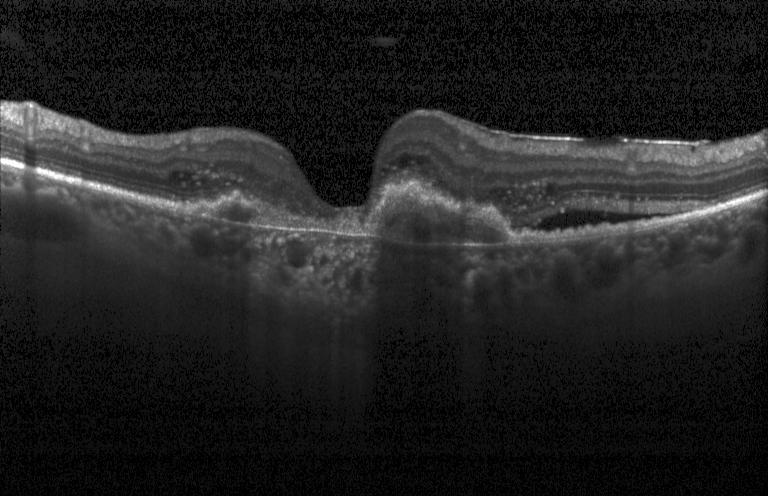
Spectral-domain OCT B-scan: choroidal neovascularization (CNV).